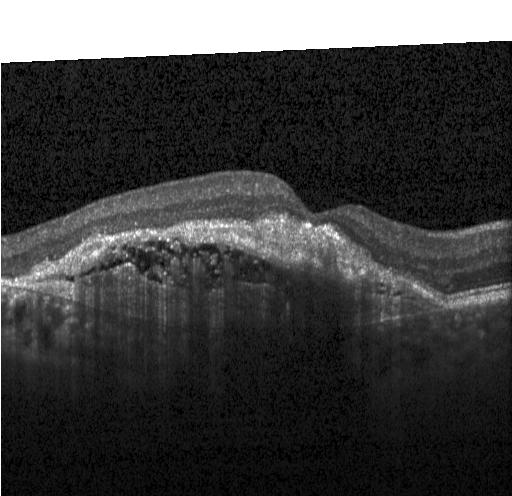

Retinal OCT B-scan
This B-scan demonstrates a choroidal neovascular membrane.